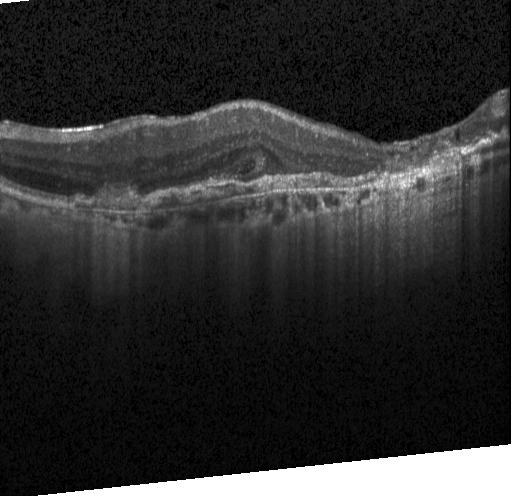

Optical coherence tomography scan
Finding: choroidal neovascularization.